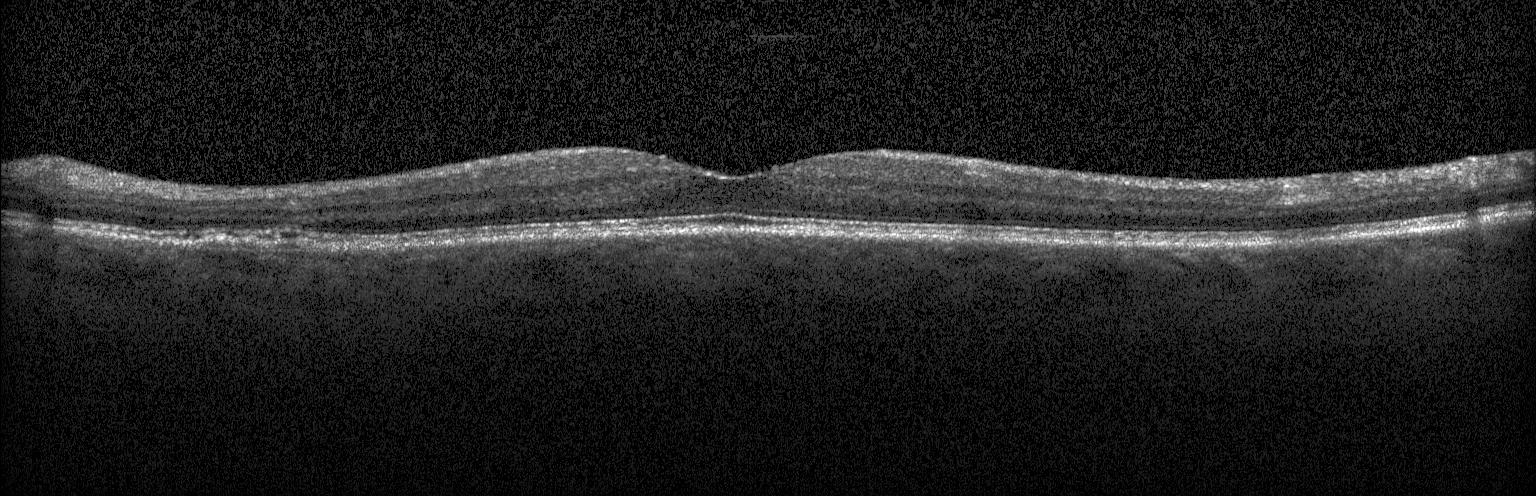 Diagnosis: choroidal neovascularization (CNV).